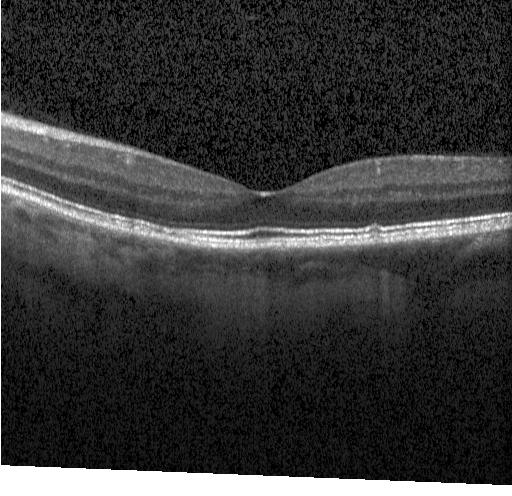 Macular scan · optical coherence tomography B-scan · instrument: Heidelberg Spectralis · spectral-domain OCT.
This B-scan demonstrates no evidence of choroidal neovascularization, diabetic macular edema, or drusen.